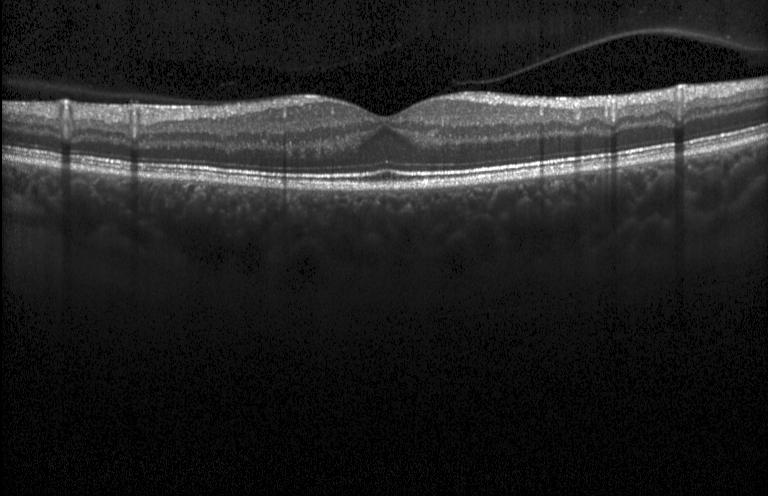

Optical coherence tomography scan · acquired on a Heidelberg Spectralis · spectral-domain OCT — Impression: neither CNV, DME, nor drusen.